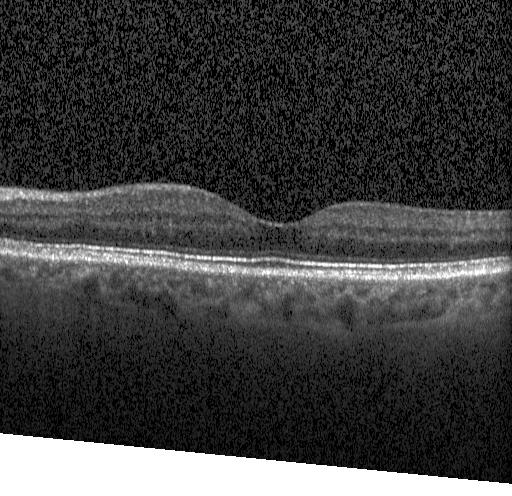 OCT finding: no choroidal neovascularization, diabetic macular edema, or drusen.